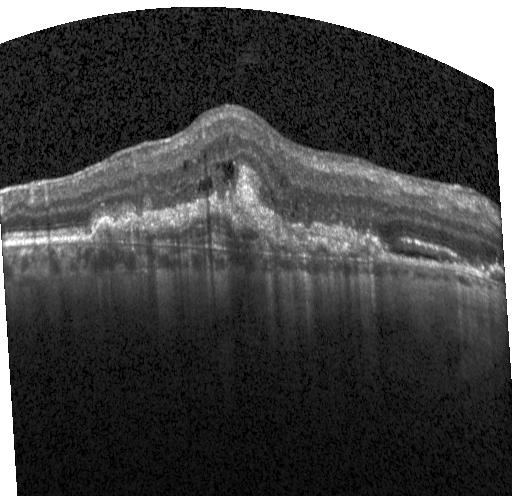
Dx: CNV.